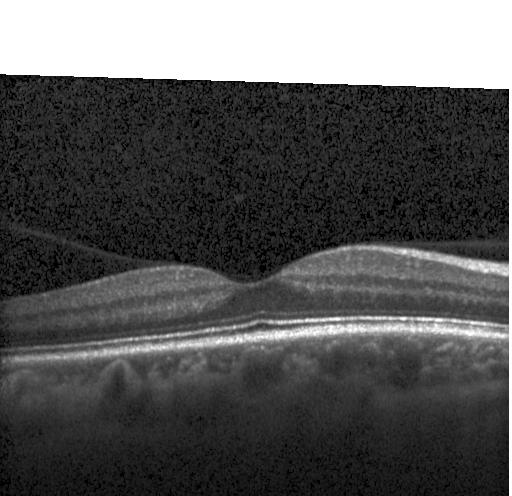

OCT B-scan
The scan shows neither CNV, DME, nor drusen.